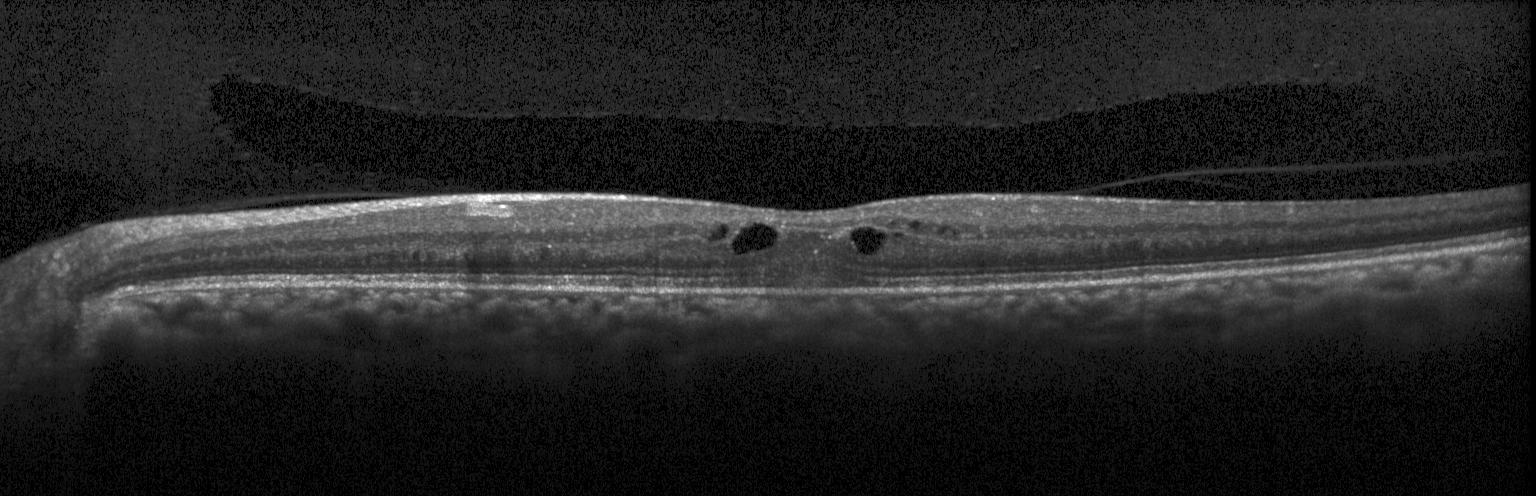
Instrument: Heidelberg Spectralis; fovea-centered; optical coherence tomography B-scan; SD-OCT.
Dx: choroidal neovascularization (CNV).